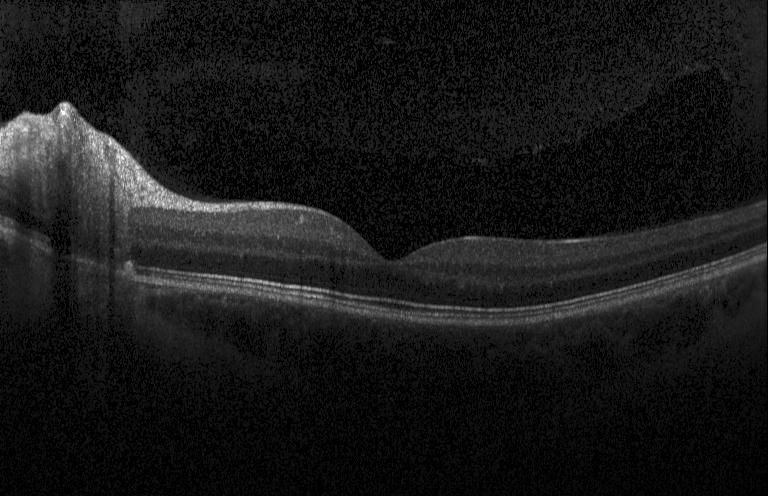

Assessment: no evidence of choroidal neovascularization, diabetic macular edema, or drusen.